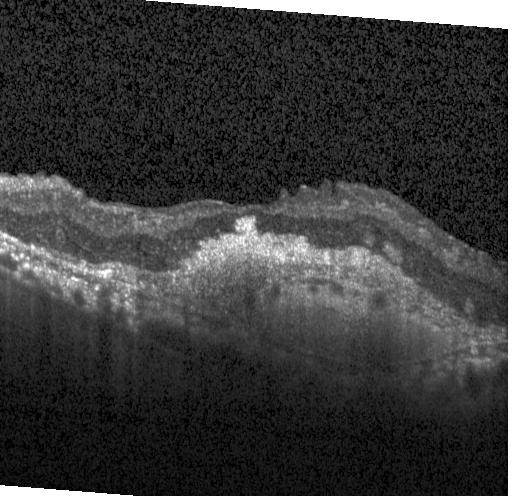 Impression: choroidal neovascularization (CNV).